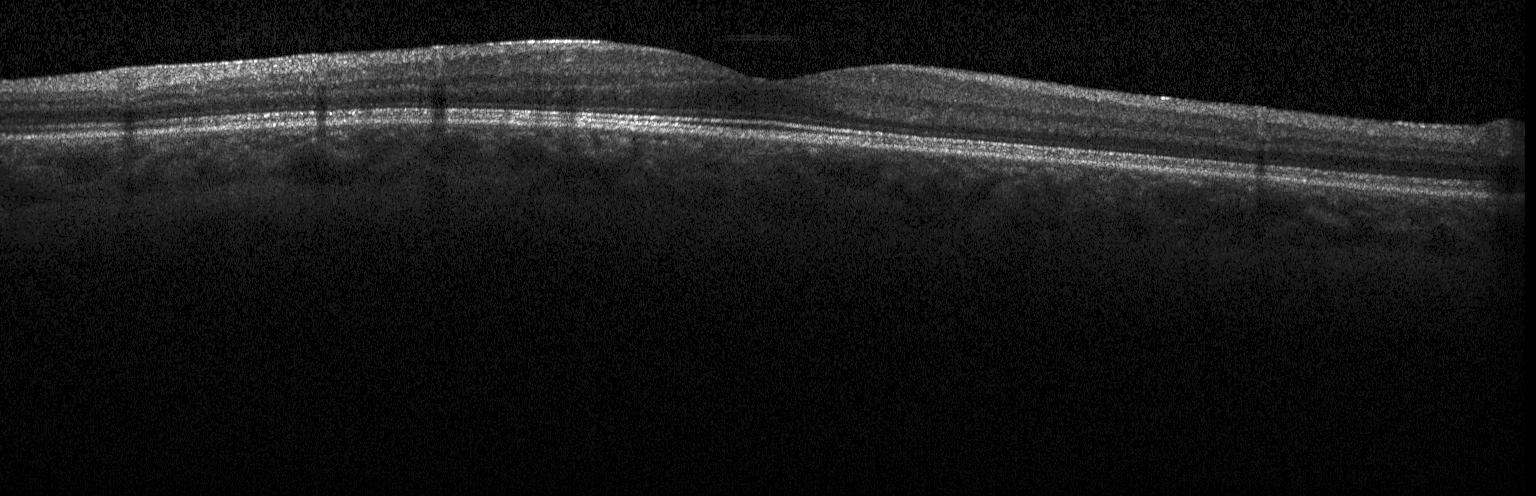
OCT line scan · instrument: Heidelberg Spectralis · SD-OCT · centered on the fovea
Finding: neither choroidal neovascularization, diabetic macular edema, nor drusen.